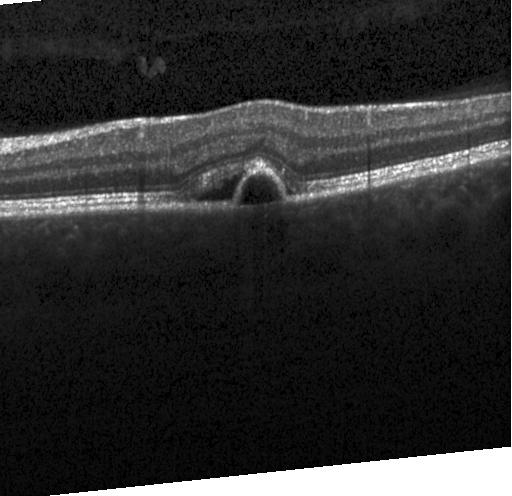

Instrument: Heidelberg Spectralis. Macular scan. Retinal OCT cross-section — Dx: a choroidal neovascular membrane.